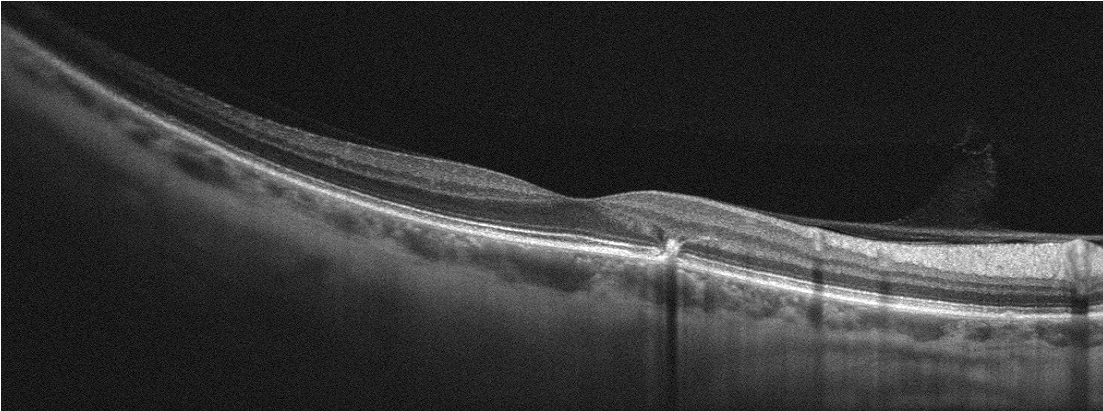

Finding: age-related macular degeneration.